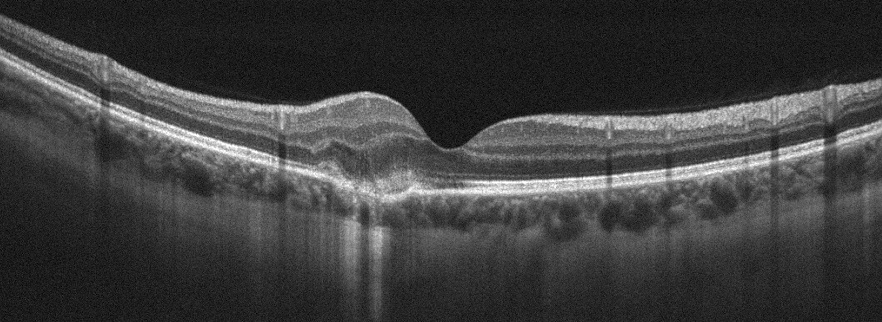

Diagnosis: AMD.